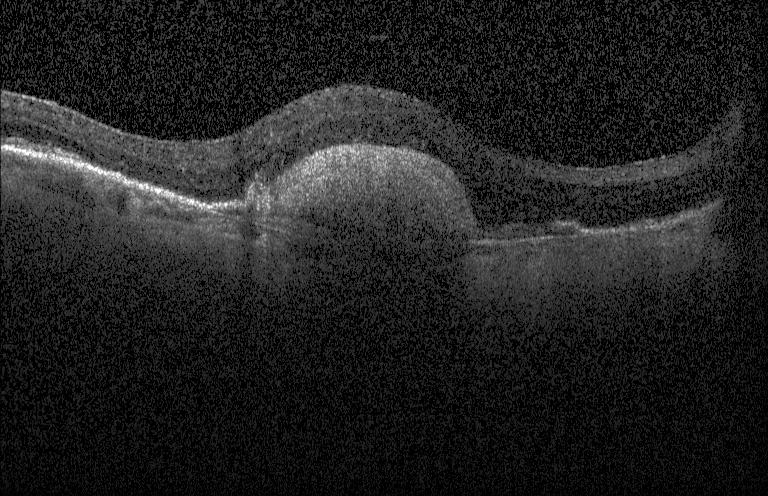 Optical coherence tomography scan.
OCT finding: a choroidal neovascular membrane.